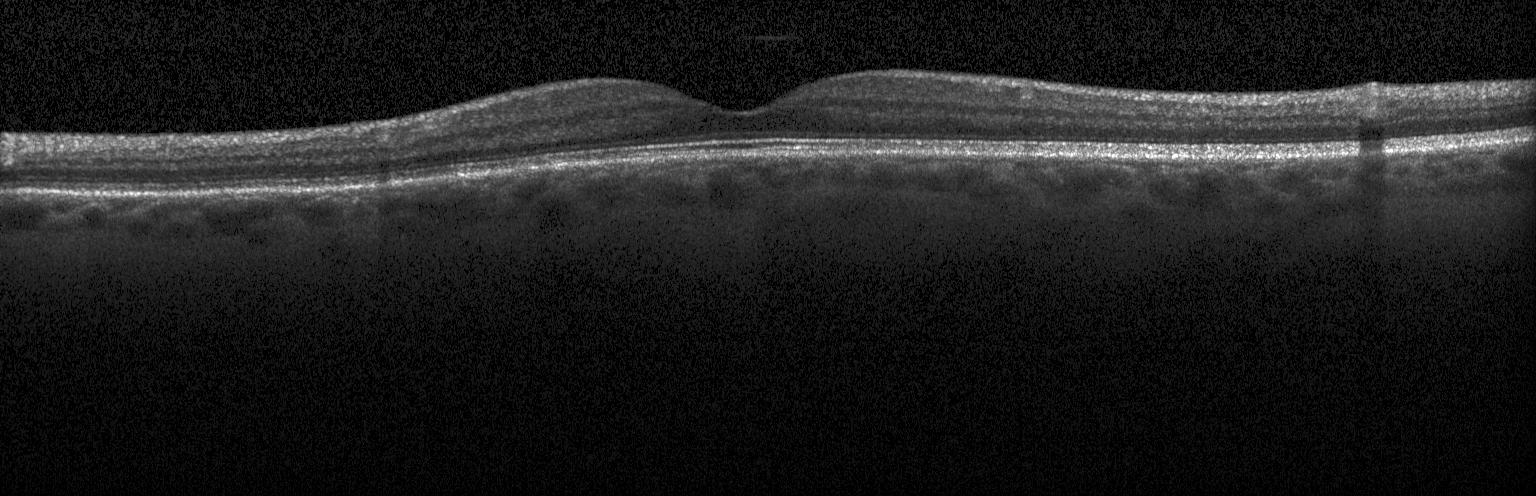 No choroidal neovascularization, no diabetic macular edema, and no drusen.